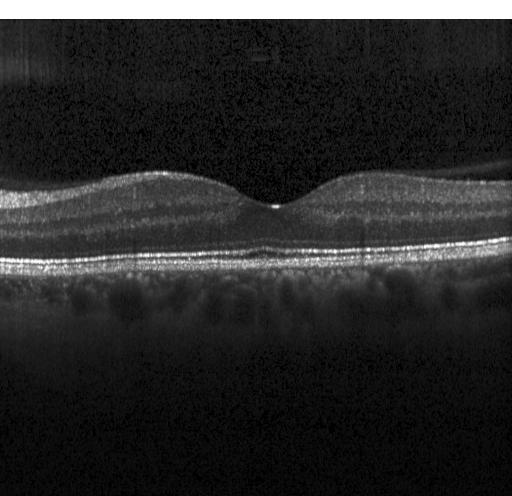

Macular scan, spectral-domain OCT, Heidelberg Spectralis, retinal OCT cross-section.
OCT finding: no CNV, DME, or drusen.